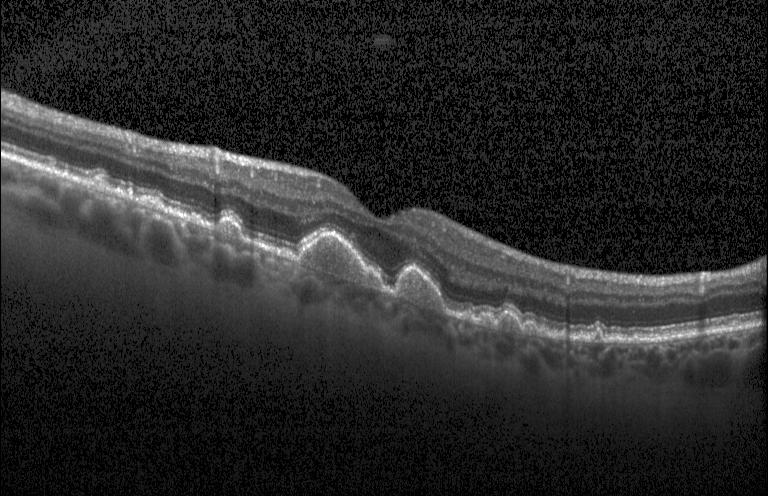
Macular scan; instrument: Heidelberg Spectralis; retinal OCT B-scan.
Multiple drusen.